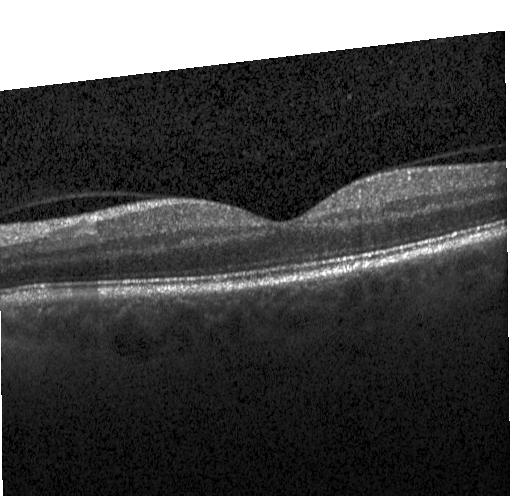
Macular OCT: neither choroidal neovascularization, diabetic macular edema, nor drusen.